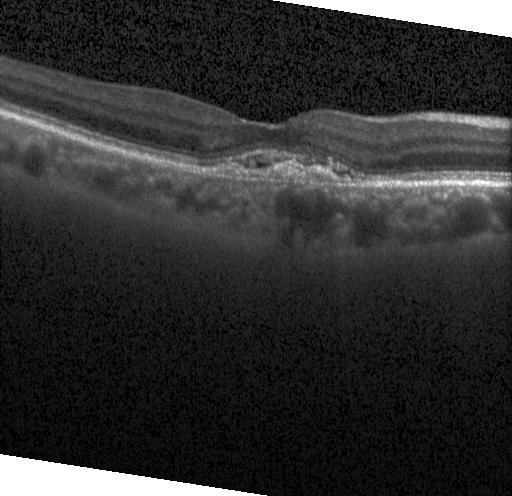

The scan shows choroidal neovascularization.